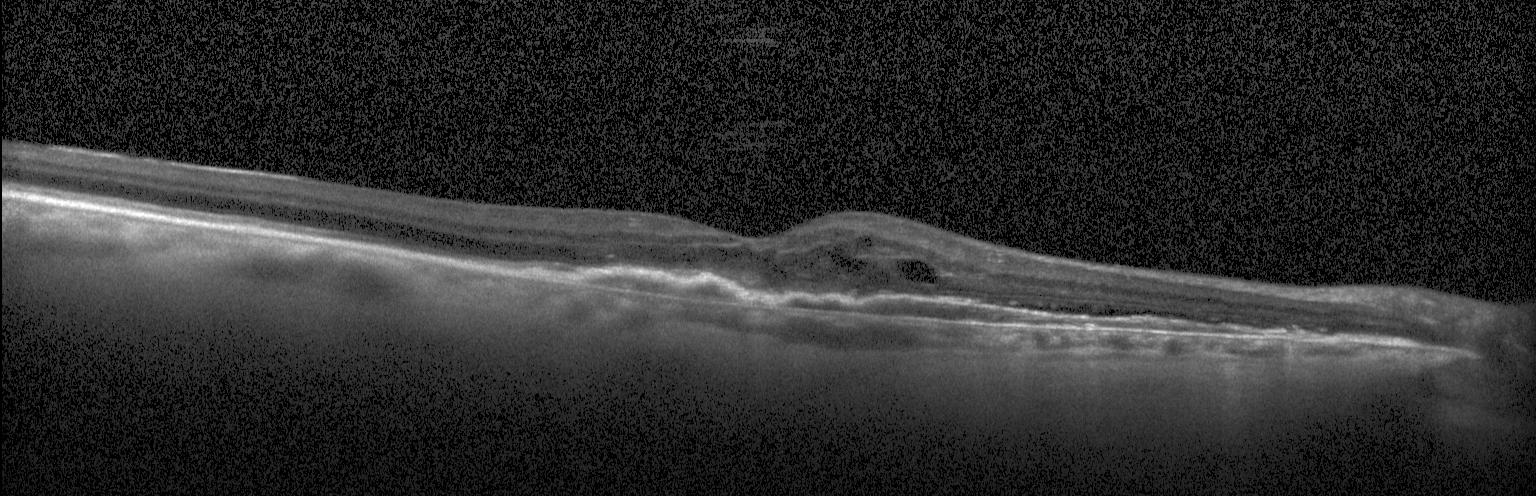
Finding: CNV.